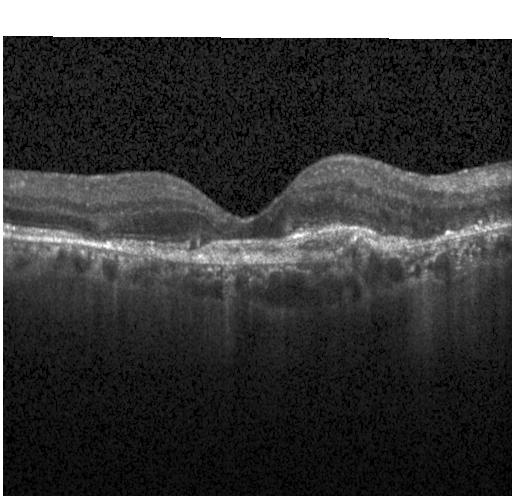
Retinal OCT cross-section — Dx: choroidal neovascularization (CNV).